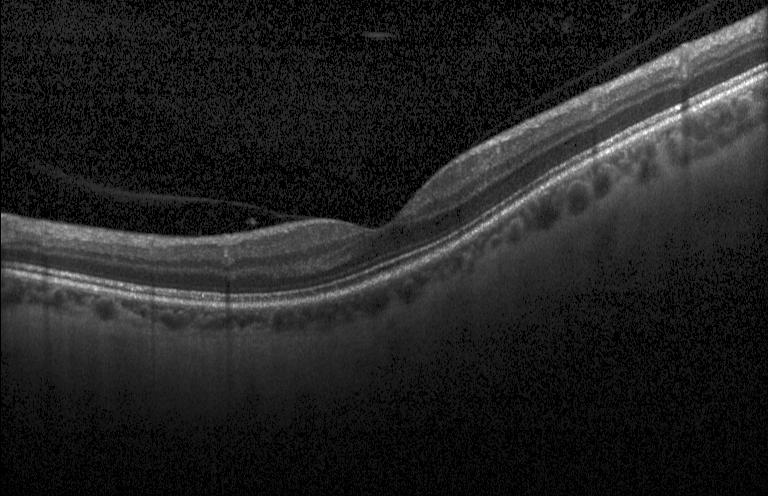
Optical coherence tomography scan.
The scan shows neither choroidal neovascularization, diabetic macular edema, nor drusen.